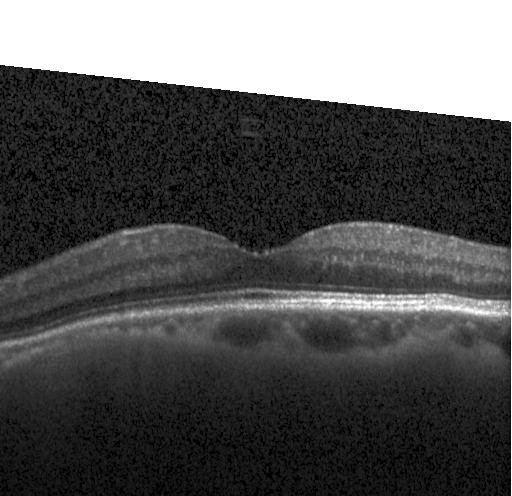

Instrument: Heidelberg Spectralis · OCT B-scan.
Impression: neither choroidal neovascularization, diabetic macular edema, nor drusen.